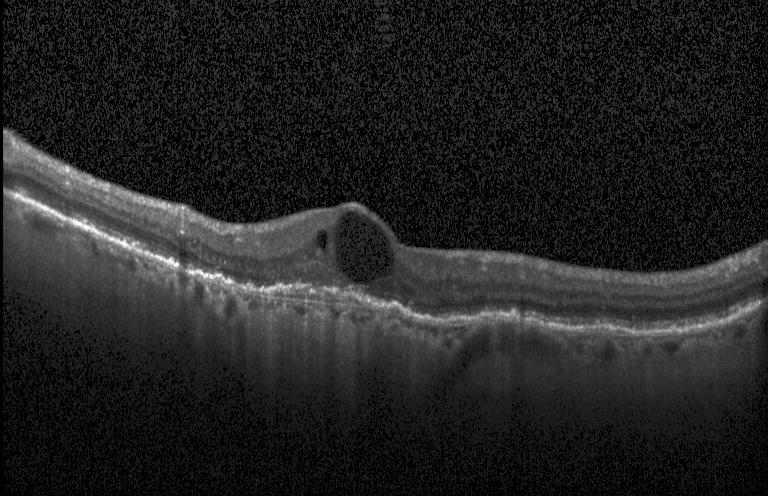

Retinal OCT B-scan · macular scan — Finding: a choroidal neovascular membrane.